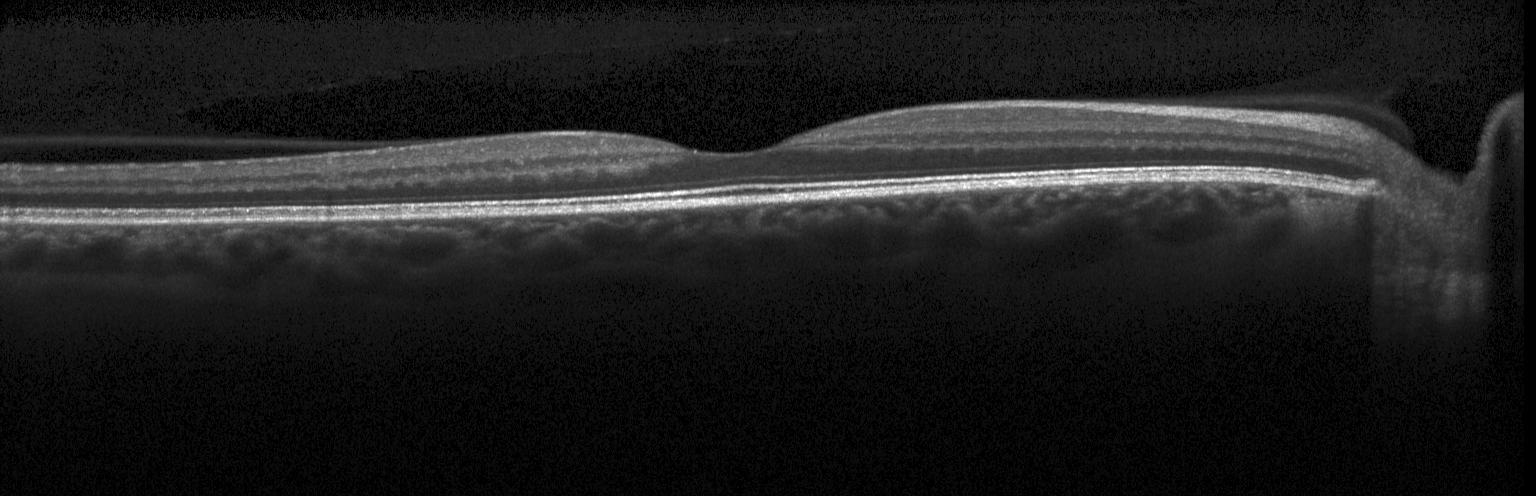

The scan shows no CNV, DME, or drusen.